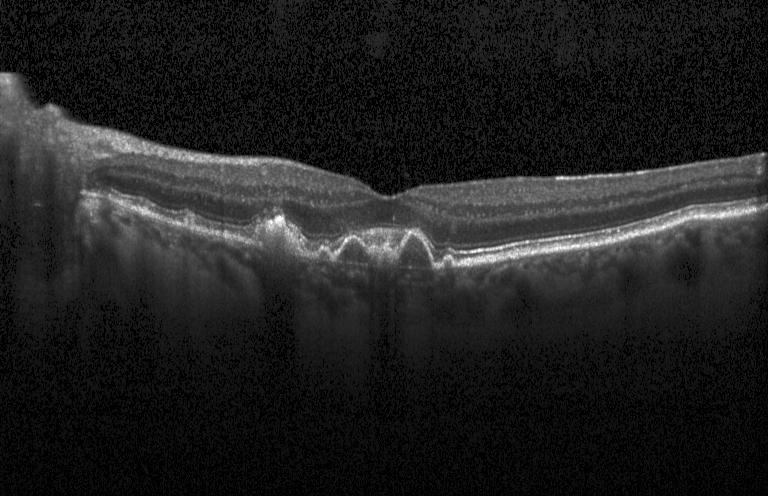
Finding: choroidal neovascularization.